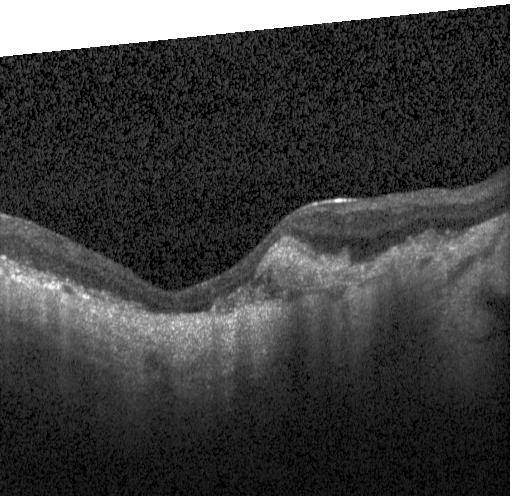

OCT line scan — Impression: CNV.